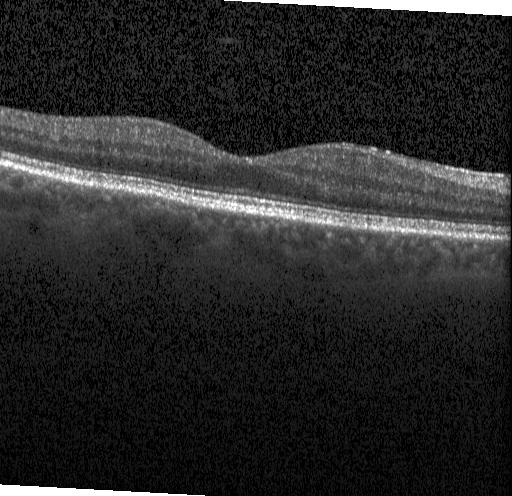
SD-OCT, retinal OCT B-scan.
Finding: neither CNV, DME, nor drusen.